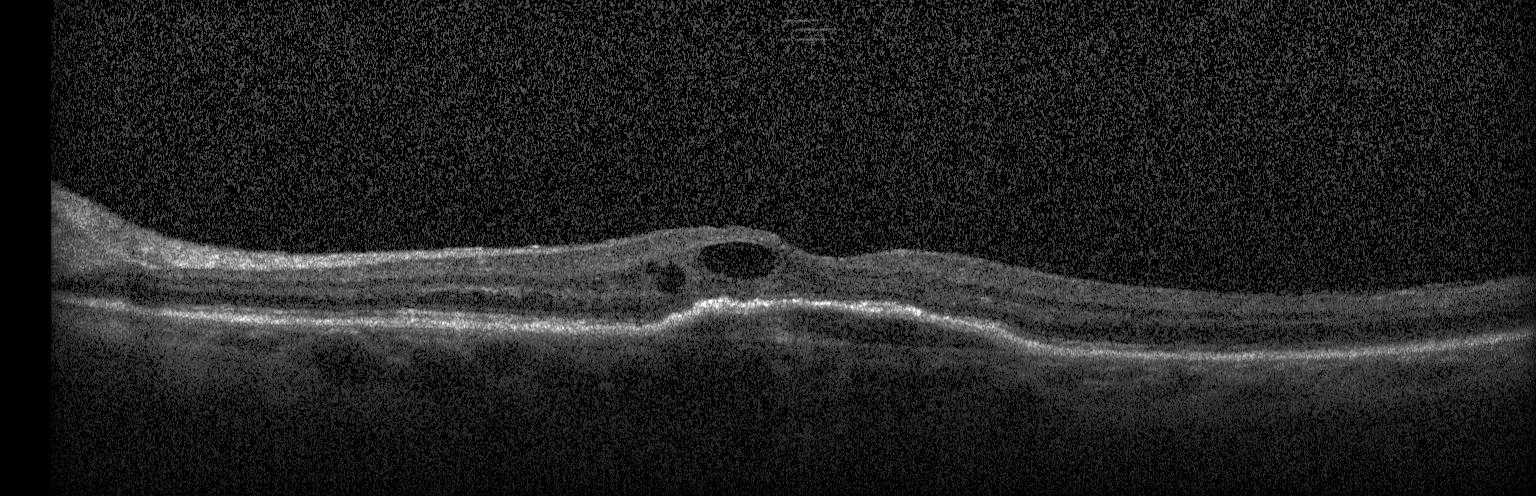
Dx: a choroidal neovascular membrane.